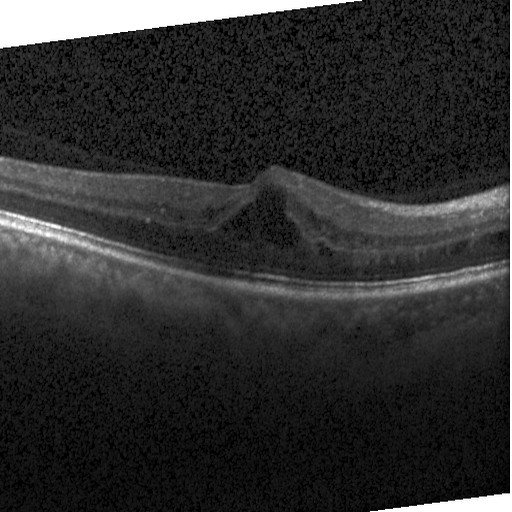

Assessment: diabetic macular edema (DME).